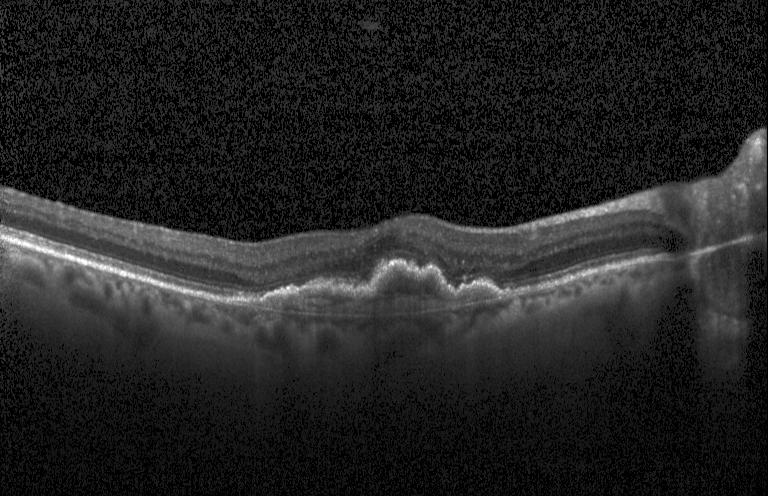 Spectral-domain OCT B-scan: a choroidal neovascular membrane.